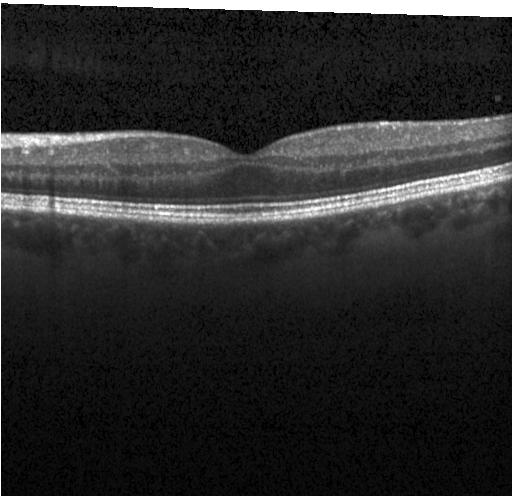
Spectral-domain OCT B-scan: no CNV, no DME, and no drusen.